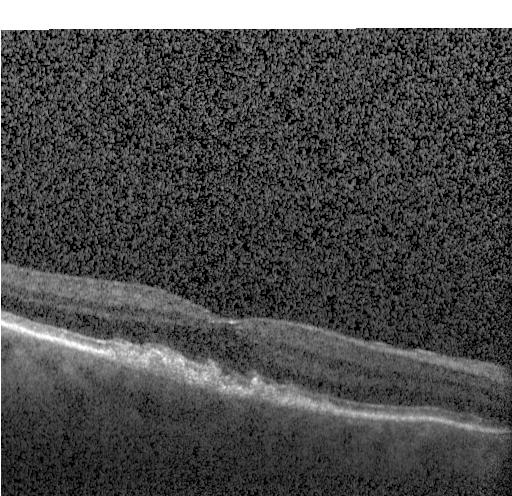

OCT B-scan, Heidelberg Spectralis OCT system. Diagnosis: sub-RPE drusenoid deposits.